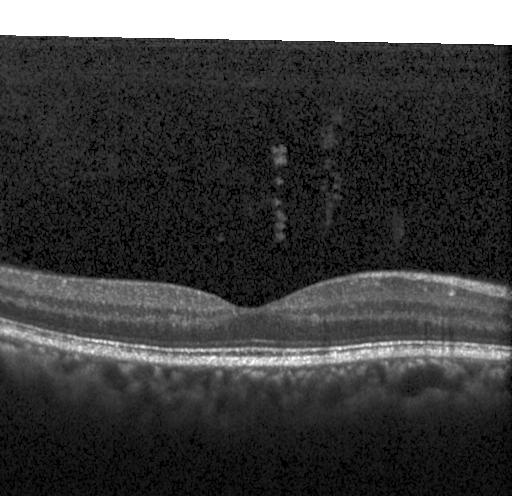
Dx: neither choroidal neovascularization, diabetic macular edema, nor drusen.